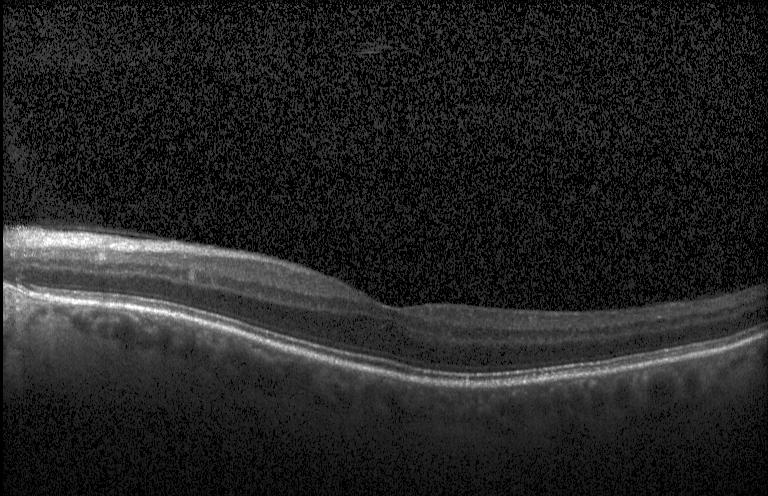 OCT finding: no CNV, DME, or drusen.